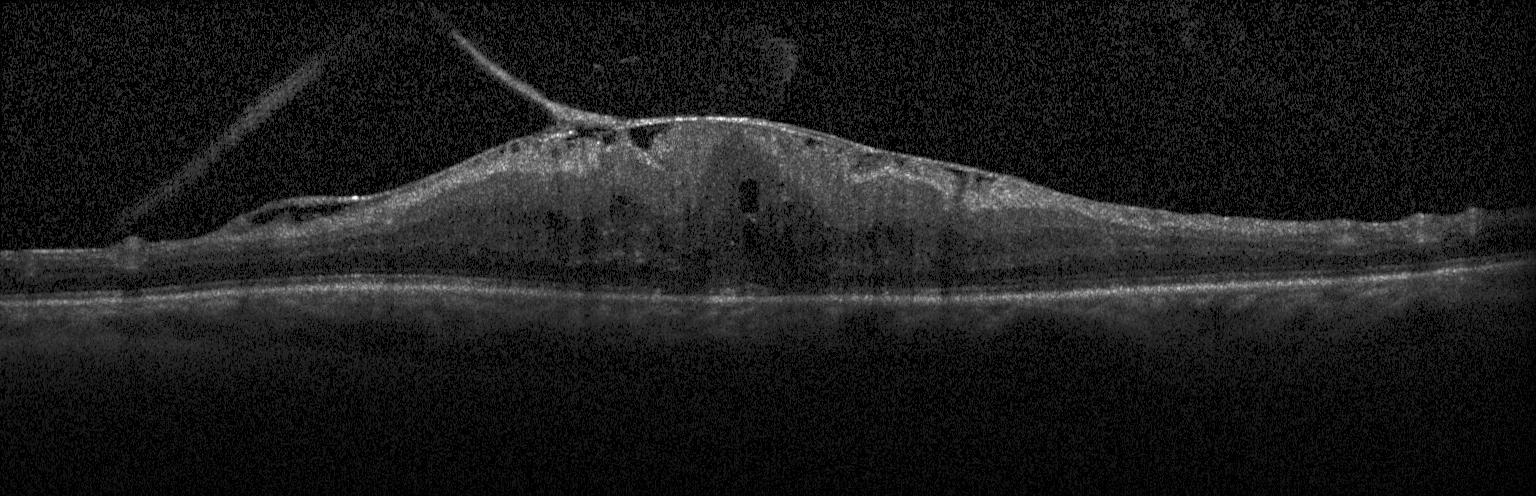

OCT line scan. Horizontal scan through the fovea — Finding: diabetic macular edema.